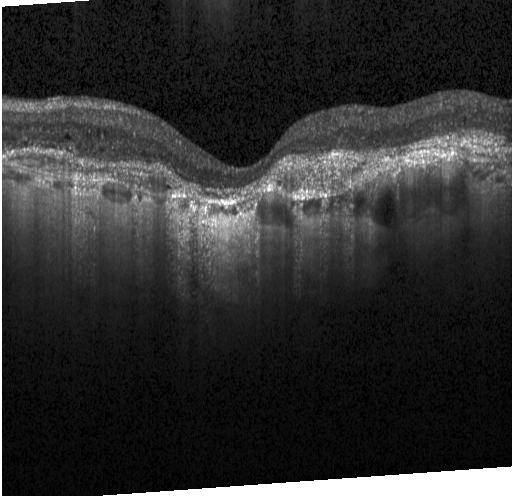

OCT finding: choroidal neovascularization.